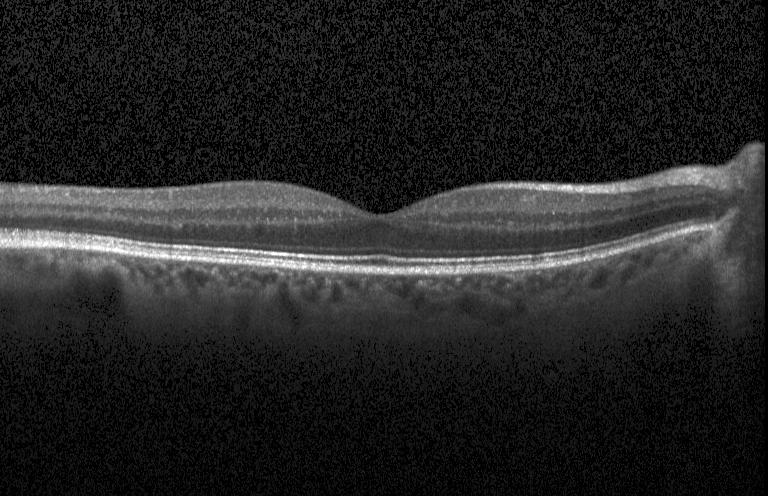
Heidelberg Spectralis OCT system, optical coherence tomography scan
Impression: neither CNV, DME, nor drusen.